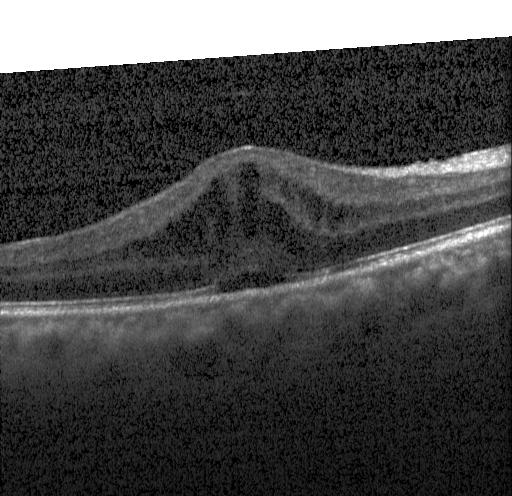
Finding: diabetic macular edema.